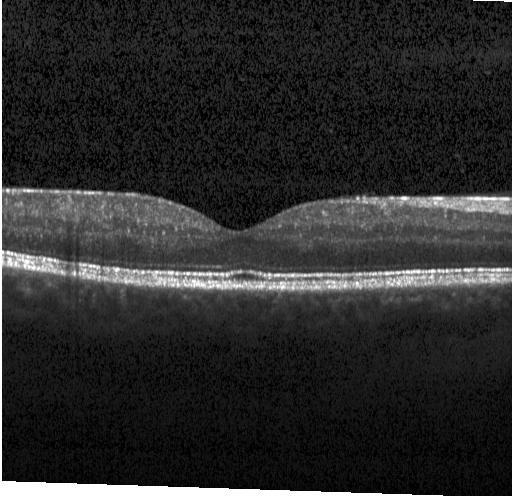
Macular OCT: no choroidal neovascularization, diabetic macular edema, or drusen.